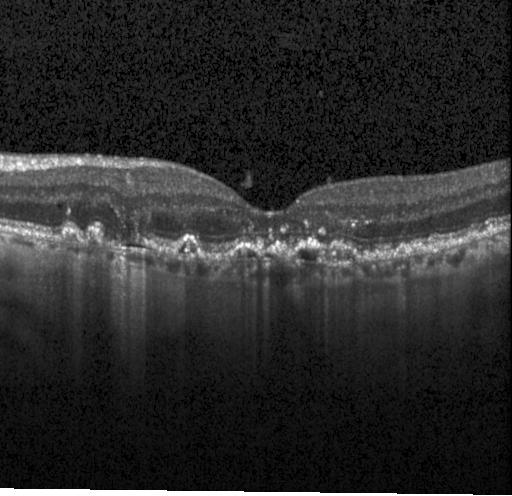
OCT line scan. Impression: choroidal neovascularization (CNV).